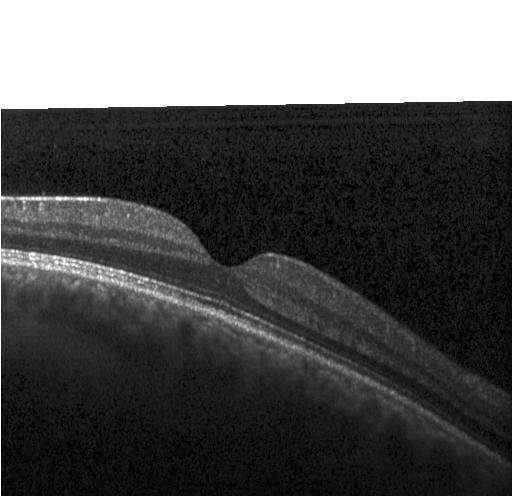

Retinal OCT B-scan.
Diagnosis: no evidence of choroidal neovascularization, diabetic macular edema, or drusen.